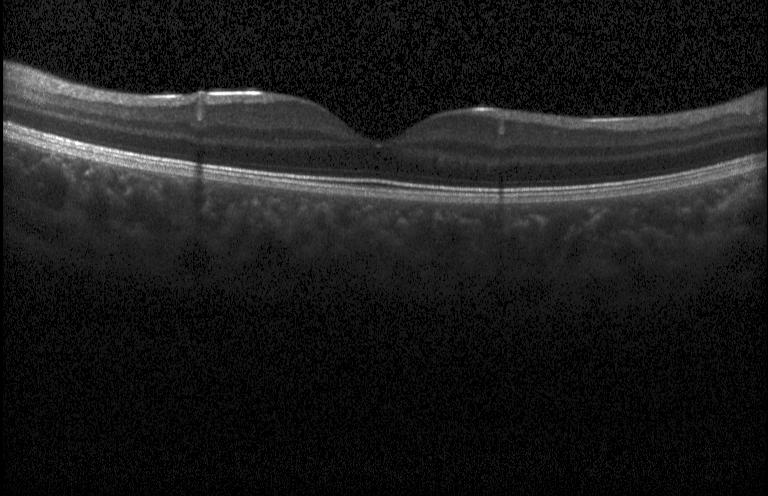
OCT B-scan; fovea-centered
OCT finding: neither choroidal neovascularization, diabetic macular edema, nor drusen.